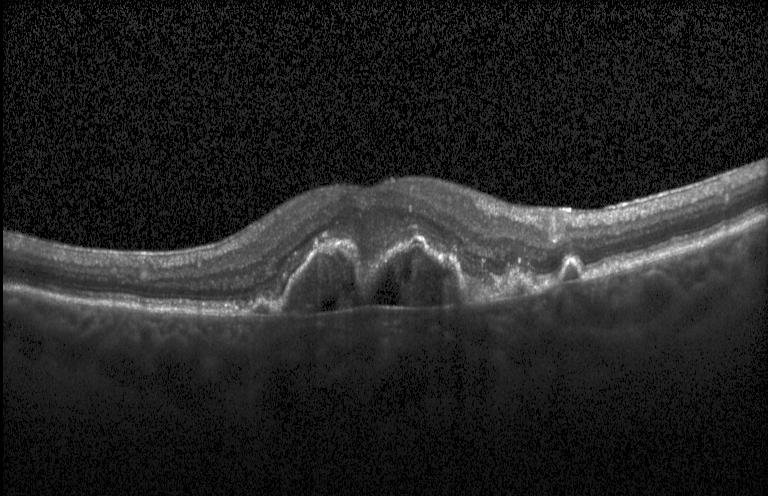

Heidelberg Spectralis, fovea-centered, retinal OCT cross-section. Finding: a choroidal neovascular membrane.